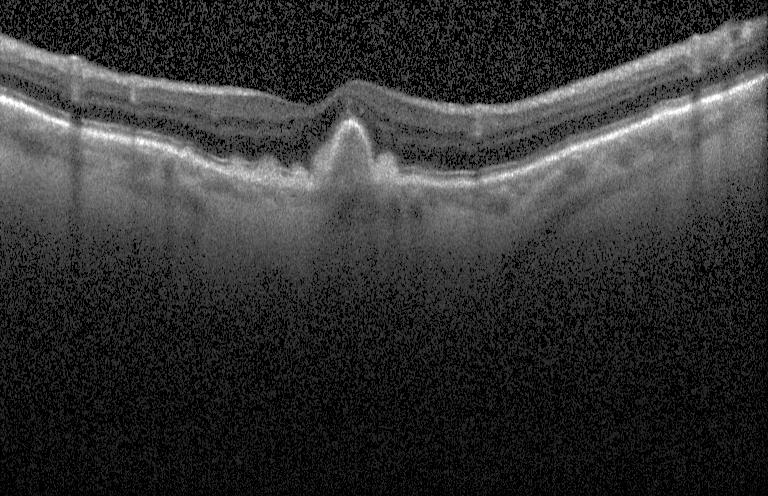

OCT line scan; instrument: Heidelberg Spectralis; macular scan; spectral-domain OCT.
Impression: multiple drusen.